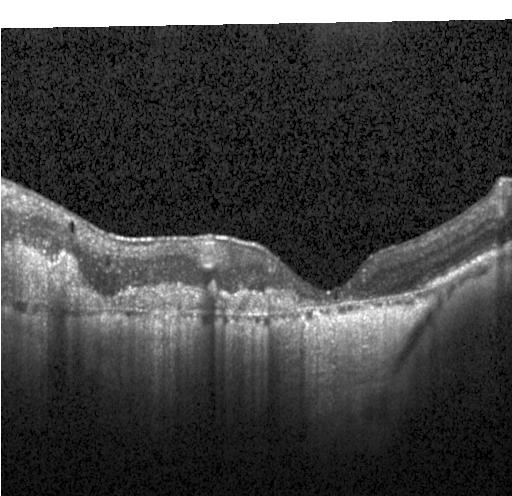

Optical coherence tomography scan. OCT finding: choroidal neovascularization (CNV).